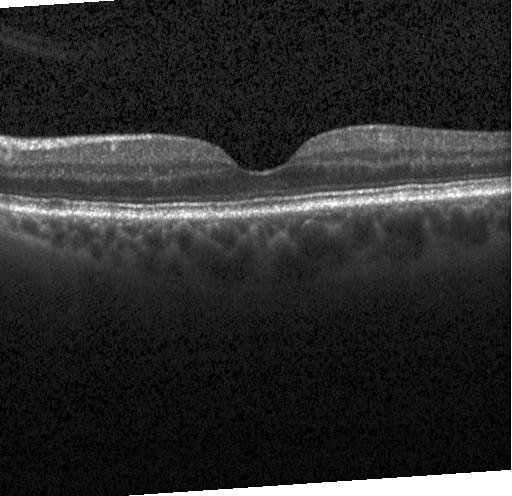 Optical coherence tomography B-scan · macular scan
Assessment: no CNV, no DME, and no drusen.